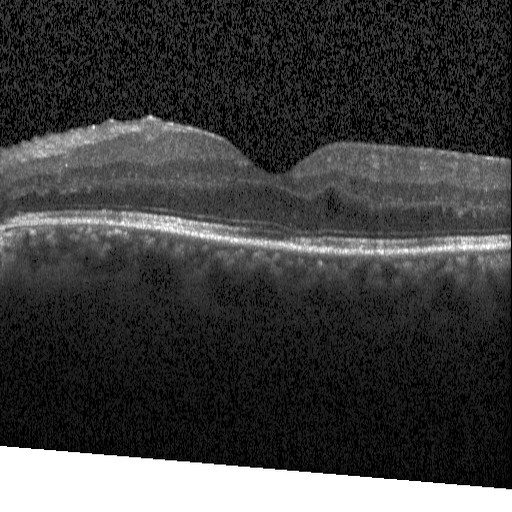

Impression: diabetic macular edema (DME).